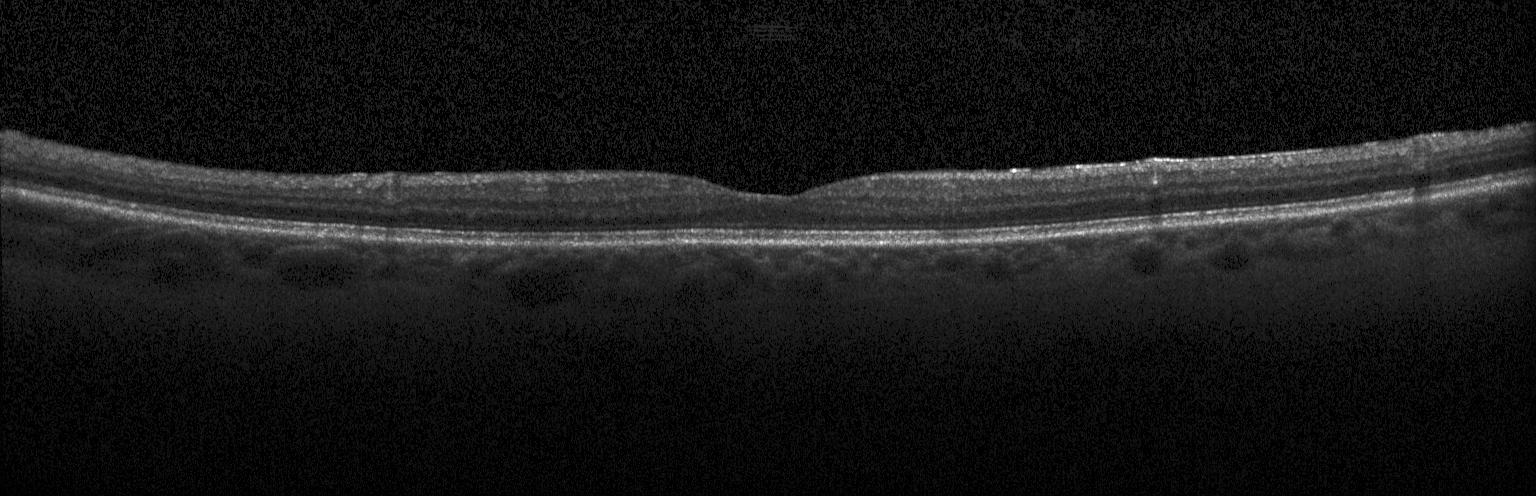

OCT finding: no evidence of choroidal neovascularization, diabetic macular edema, or drusen.